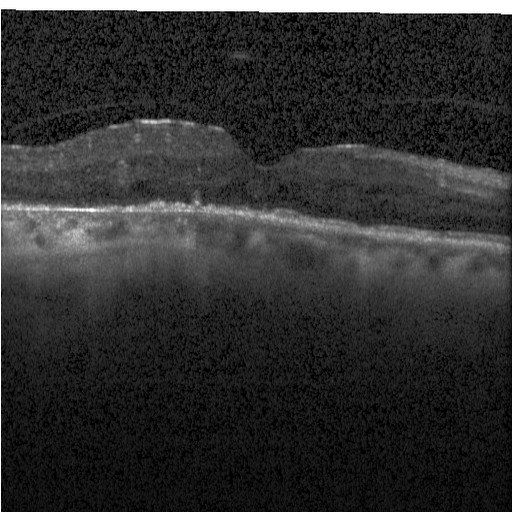
Retinal OCT B-scan; centered on the fovea — OCT finding: diabetic macular edema (DME).